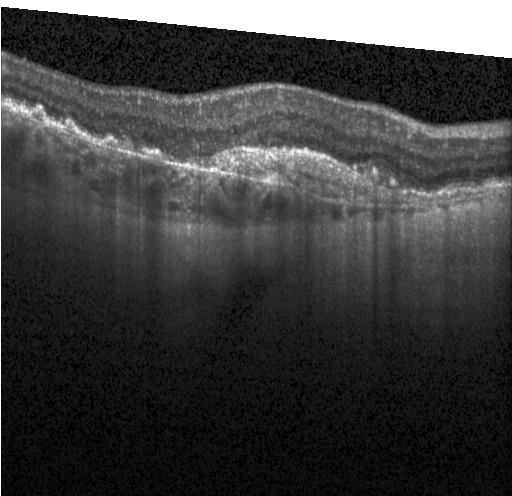

Optical coherence tomography scan
Macular OCT: choroidal neovascularization.